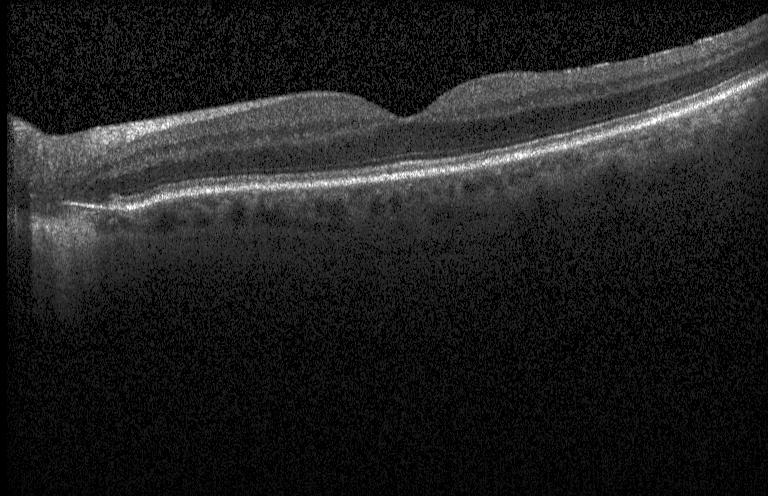

Through the macula; optical coherence tomography B-scan — Impression: no choroidal neovascularization, no diabetic macular edema, and no drusen.